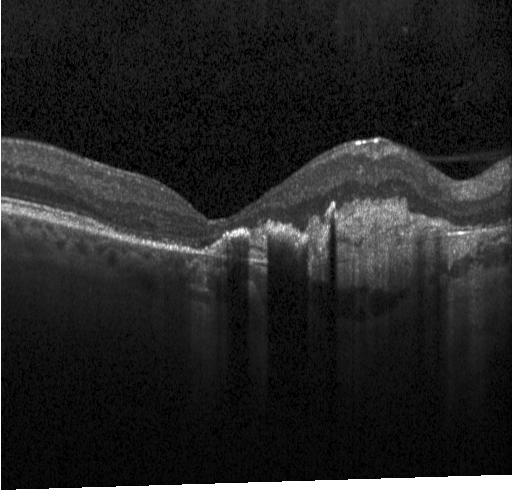 Optical coherence tomography B-scan
Finding: a choroidal neovascular membrane.